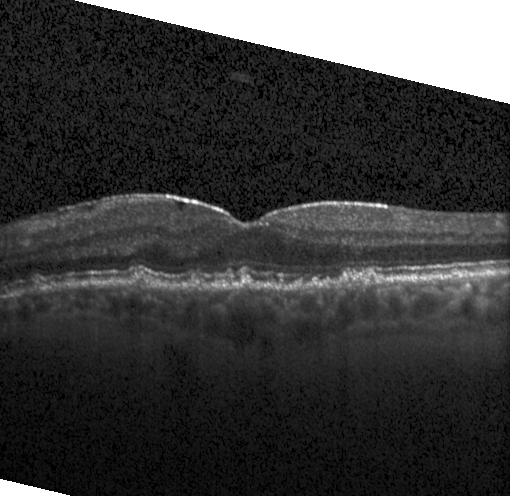 Heidelberg Spectralis OCT system. Optical coherence tomography scan
Impression: sub-RPE drusenoid deposits.